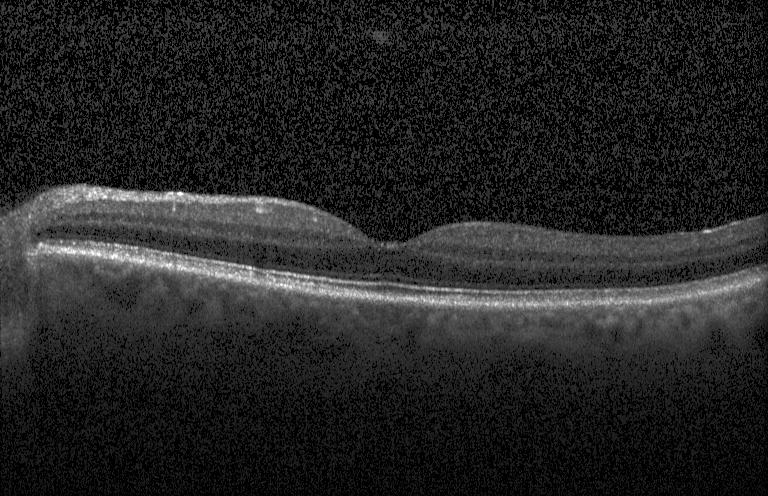 Retinal OCT B-scan. The scan shows no choroidal neovascularization, no diabetic macular edema, and no drusen.